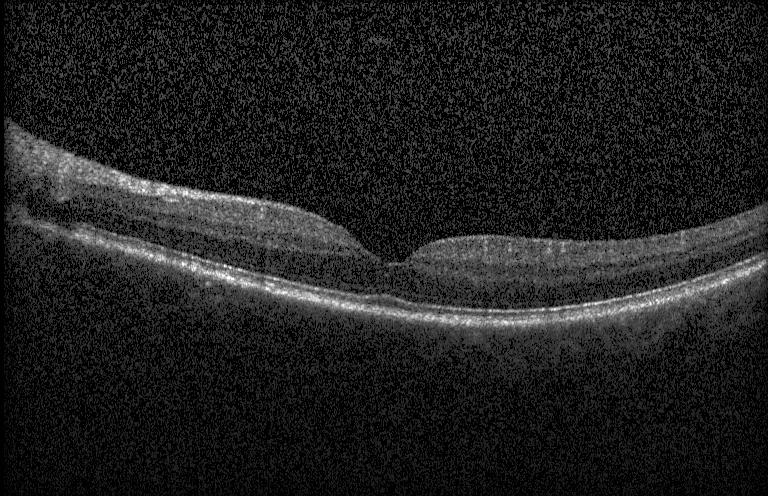

Centered on the fovea. Optical coherence tomography scan. OCT finding: no choroidal neovascularization, diabetic macular edema, or drusen.